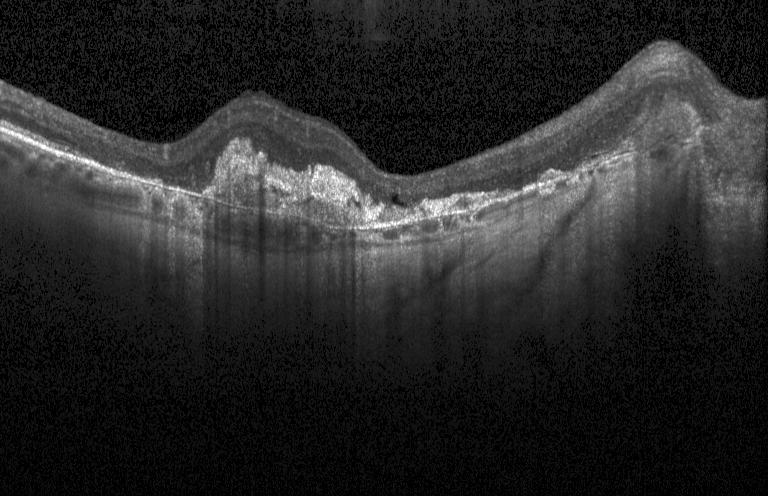 Optical coherence tomography scan.
OCT finding: a choroidal neovascular membrane.